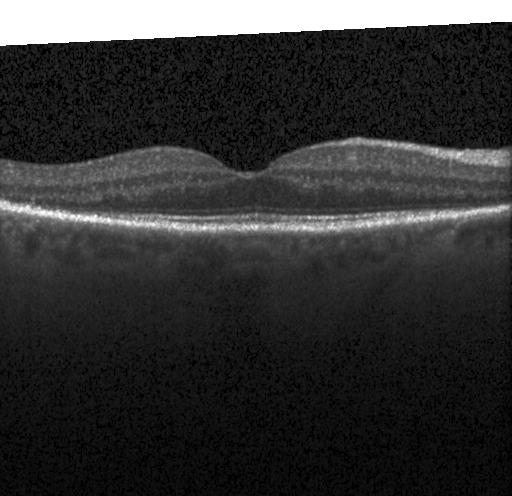

Through the macula, optical coherence tomography B-scan, Heidelberg Spectralis OCT system, spectral-domain OCT.
The scan shows no evidence of choroidal neovascularization, diabetic macular edema, or drusen.